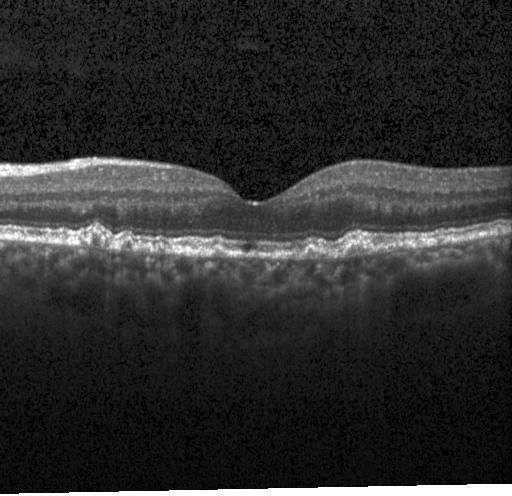 Spectral-domain OCT · instrument: Heidelberg Spectralis · retinal OCT B-scan — The scan shows multiple drusen.